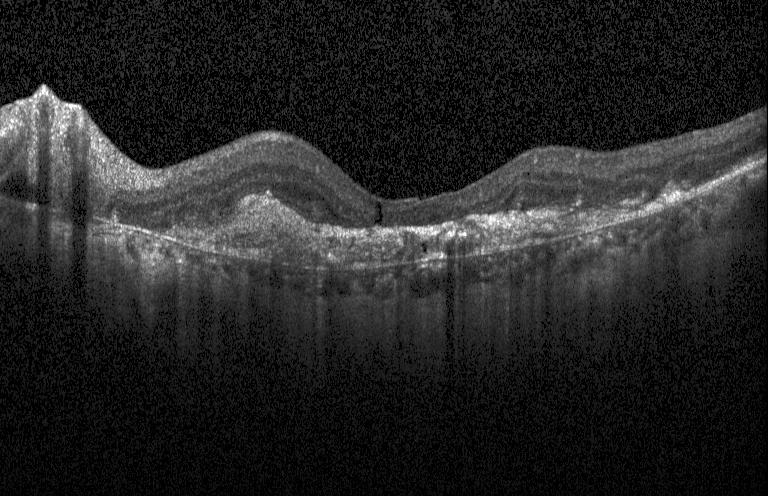 Horizontal scan through the fovea, retinal OCT B-scan, acquired on a Heidelberg Spectralis — Finding: a choroidal neovascular membrane.